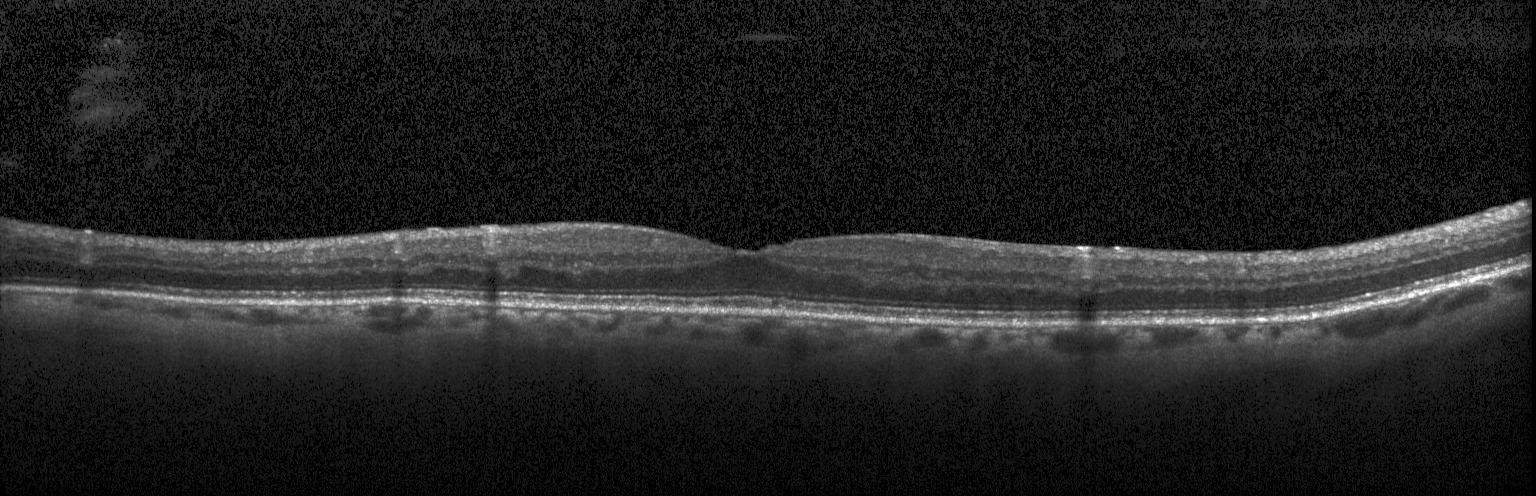 OCT line scan. Horizontal scan through the fovea. Heidelberg Spectralis.
The scan shows no choroidal neovascularization, diabetic macular edema, or drusen.